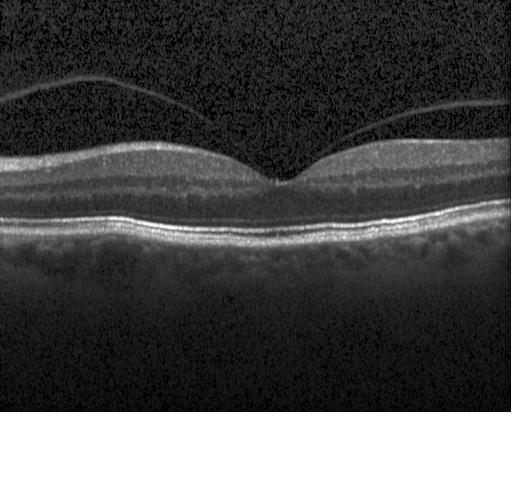 Retinal OCT cross-section. Spectral-domain OCT. Fovea-centered.
Macular OCT: no CNV, DME, or drusen.